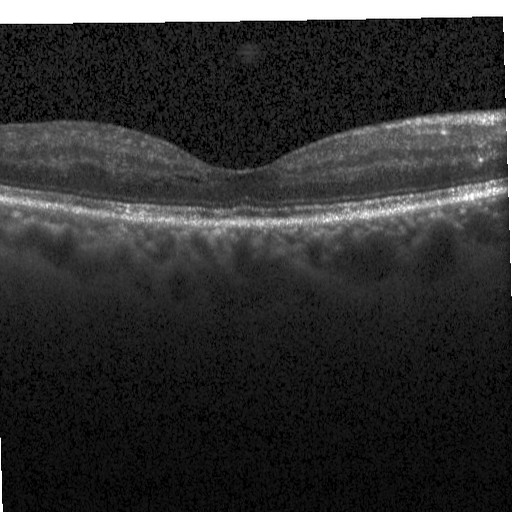

Acquired on a Heidelberg Spectralis · OCT line scan · spectral-domain OCT.
Finding: diabetic macular edema (DME).